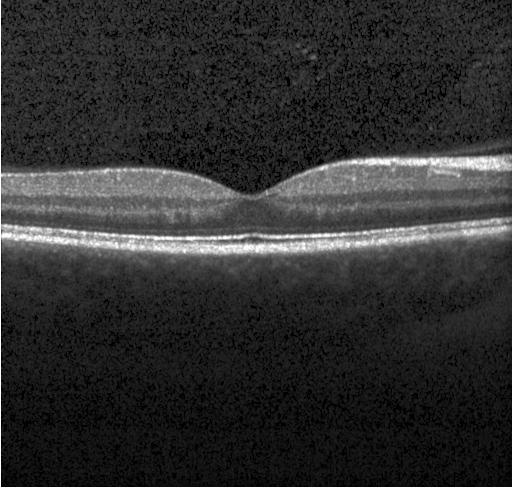
Finding: no evidence of choroidal neovascularization, diabetic macular edema, or drusen.